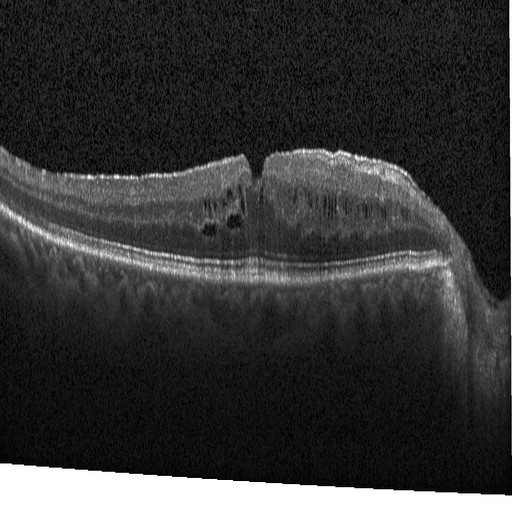

SD-OCT. Optical coherence tomography B-scan. Through the macula. Heidelberg Spectralis.
Diagnosis: DME.